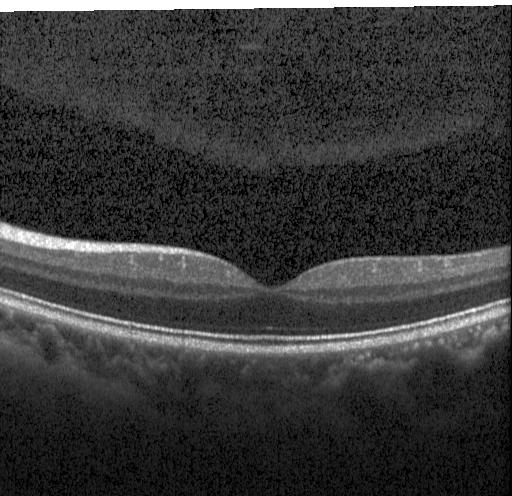
Optical coherence tomography B-scan.
Finding: no choroidal neovascularization, no diabetic macular edema, and no drusen.